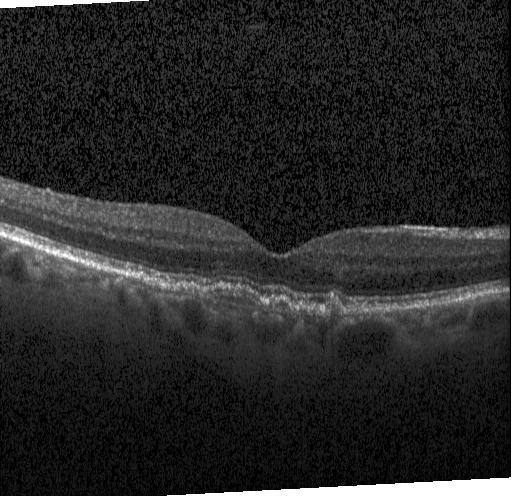

Retinal OCT cross-section. Acquired on a Heidelberg Spectralis
Impression: a choroidal neovascular membrane.